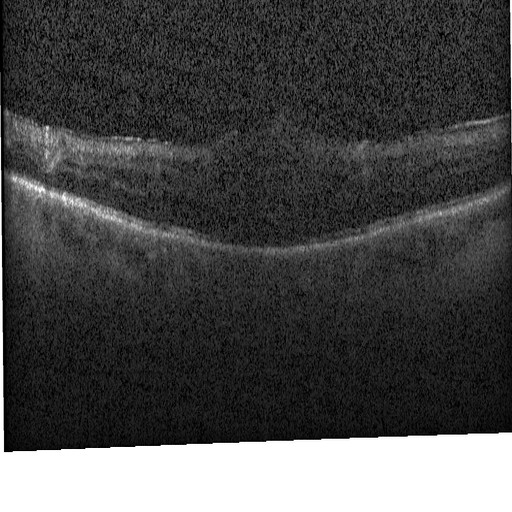
Optical coherence tomography B-scan; spectral-domain OCT; acquired on a Heidelberg Spectralis; centered on the fovea
Diagnosis: diabetic macular edema (DME).